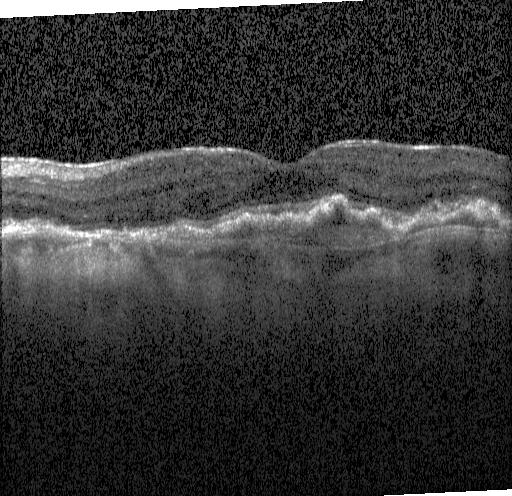 Retinal OCT B-scan; through the macula — Finding: CNV.